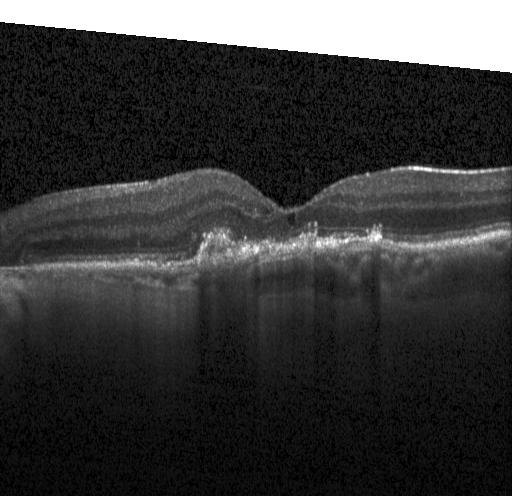

OCT B-scan — Impression: a choroidal neovascular membrane.